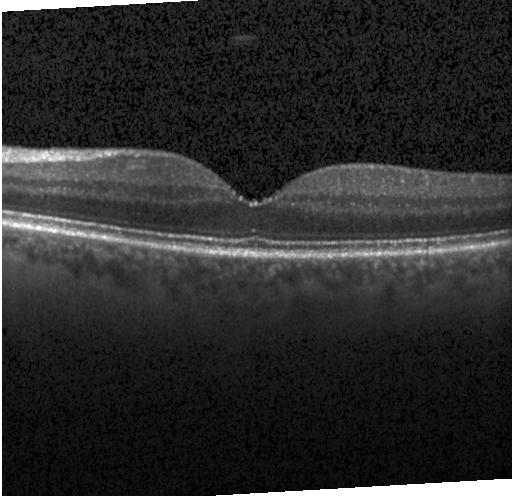 The scan shows no evidence of CNV, DME, or drusen.